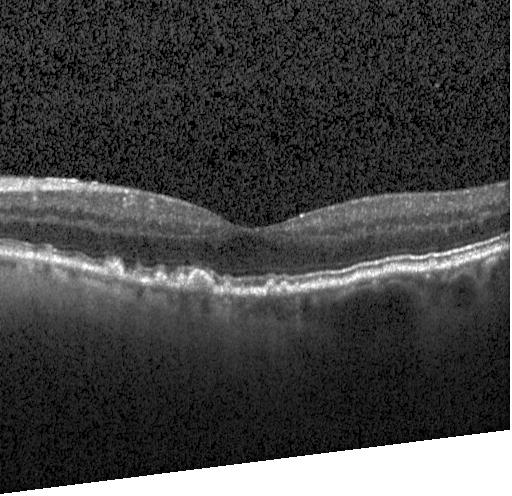 Optical coherence tomography scan
Diagnosis: multiple drusen.